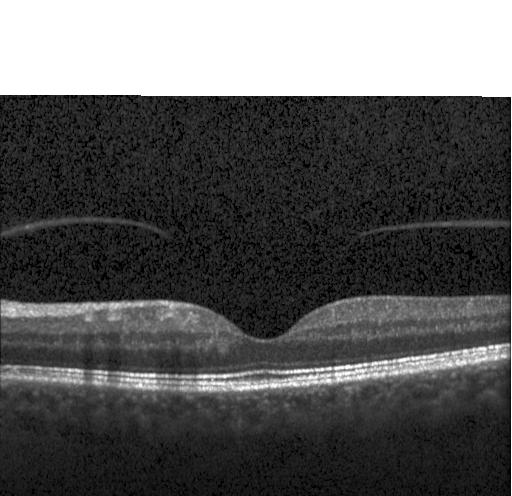

Optical coherence tomography B-scan — The scan shows no CNV, no DME, and no drusen.